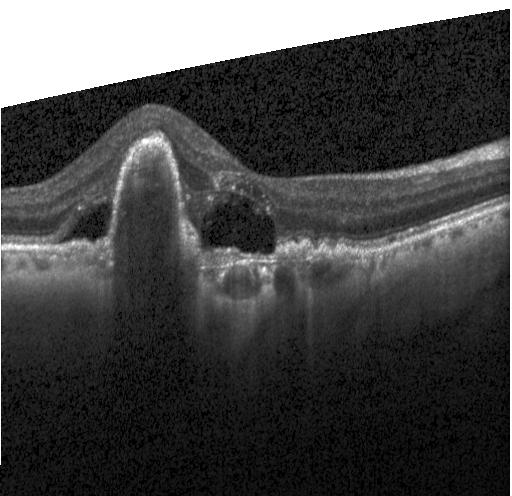

OCT scan showing CNV.